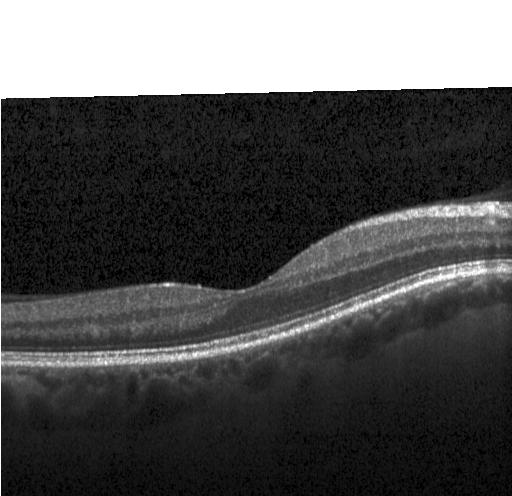
OCT B-scan; fovea-centered. Macular OCT: neither choroidal neovascularization, diabetic macular edema, nor drusen.